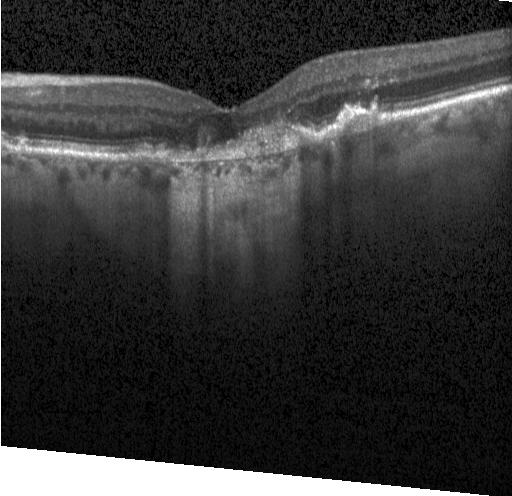 Spectral-domain OCT B-scan: CNV.